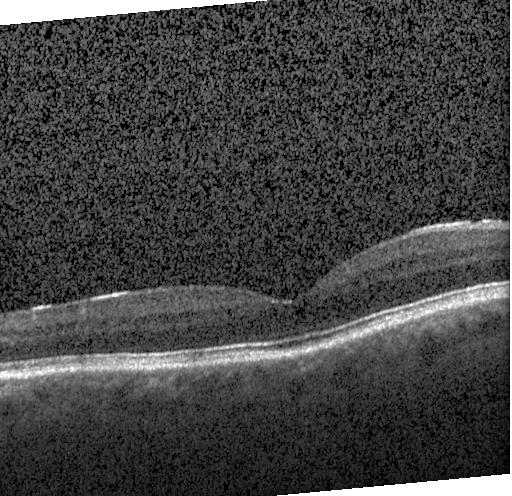
OCT B-scan.
This B-scan demonstrates neither CNV, DME, nor drusen.